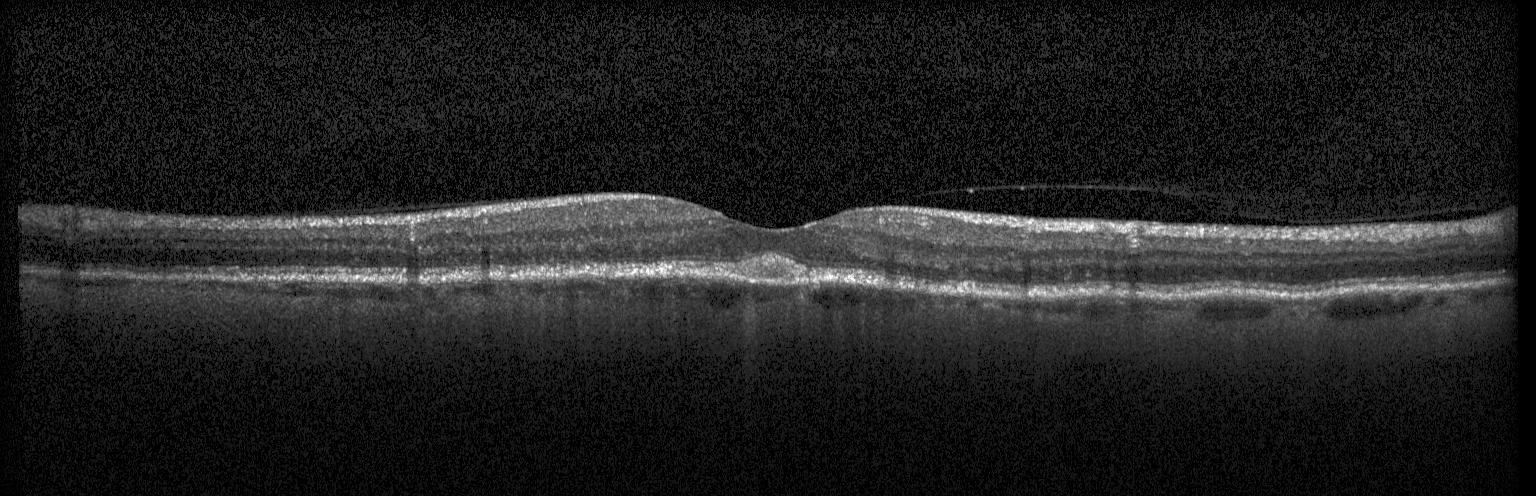

Retinal OCT B-scan; fovea-centered; spectral-domain optical coherence tomography — Macular OCT: multiple drusen.